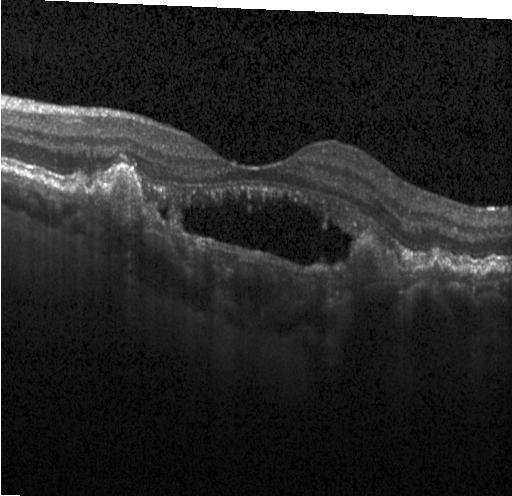 Retinal OCT cross-section. The scan shows choroidal neovascularization.